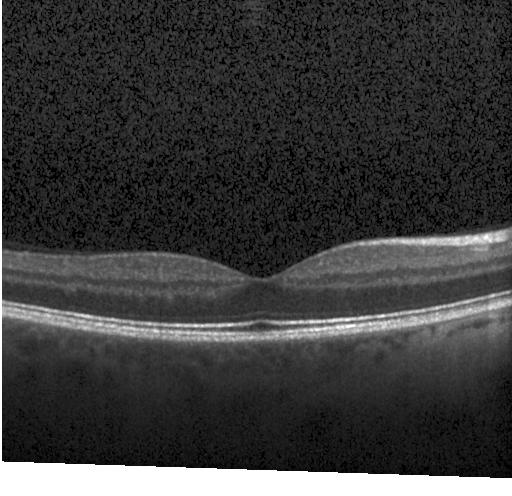 Retinal OCT B-scan · instrument: Heidelberg Spectralis · spectral-domain OCT · macular scan.
Macular OCT: neither choroidal neovascularization, diabetic macular edema, nor drusen.